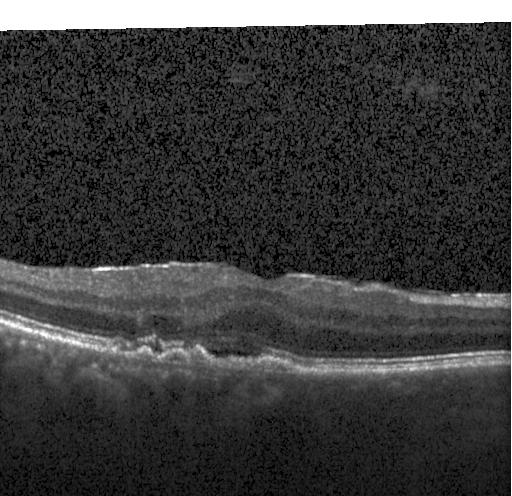

OCT scan showing choroidal neovascularization.